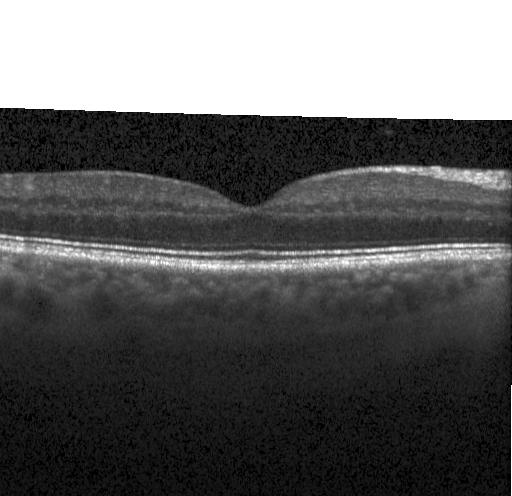
Through the macula · OCT line scan · Heidelberg Spectralis. Macular OCT: no evidence of CNV, DME, or drusen.